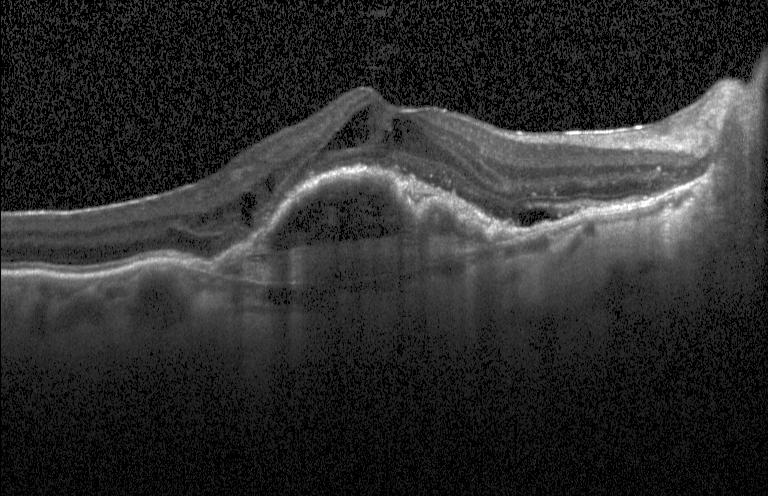

OCT B-scan. Spectral-domain optical coherence tomography
Diagnosis: choroidal neovascularization (CNV).